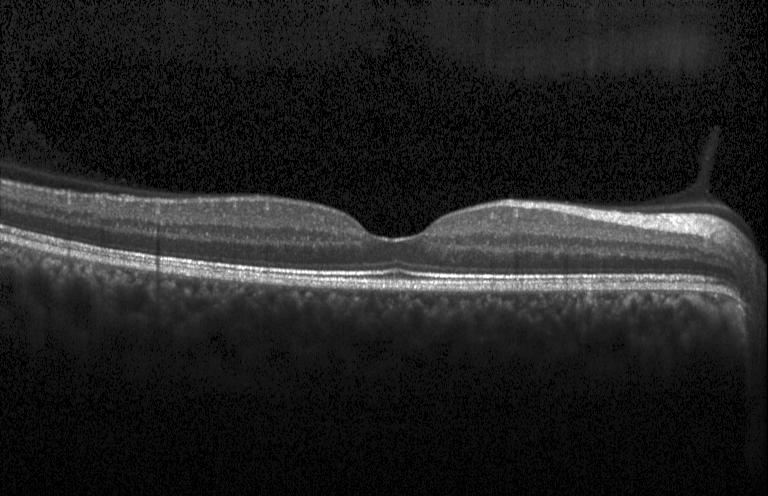
Centered on the fovea · SD-OCT · optical coherence tomography scan.
Diagnosis: no choroidal neovascularization, diabetic macular edema, or drusen.